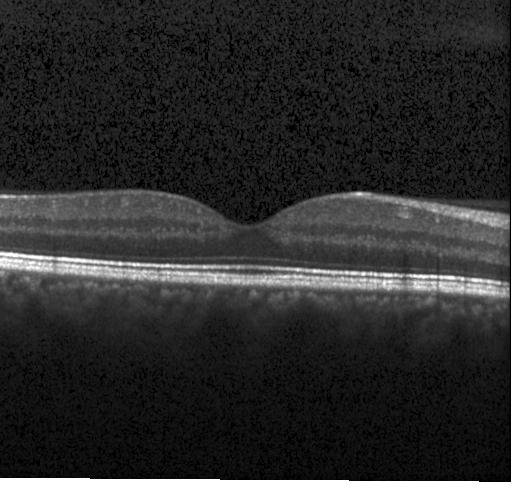
OCT line scan. Acquired on a Heidelberg Spectralis.
Diagnosis: no choroidal neovascularization, diabetic macular edema, or drusen.